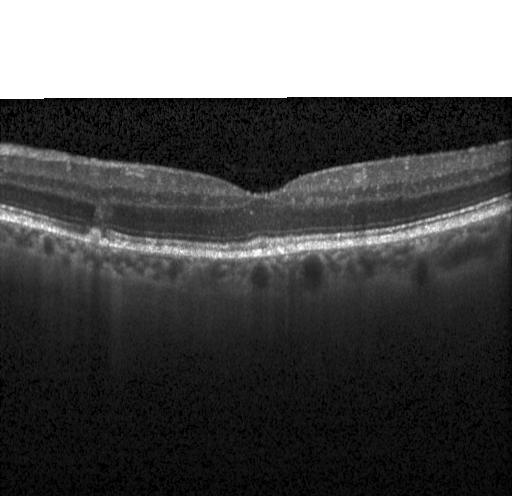 OCT finding: drusen.